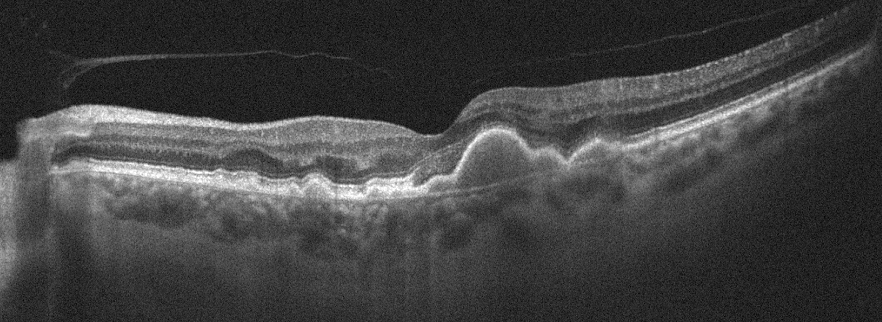

Dx: age-related macular degeneration (AMD).